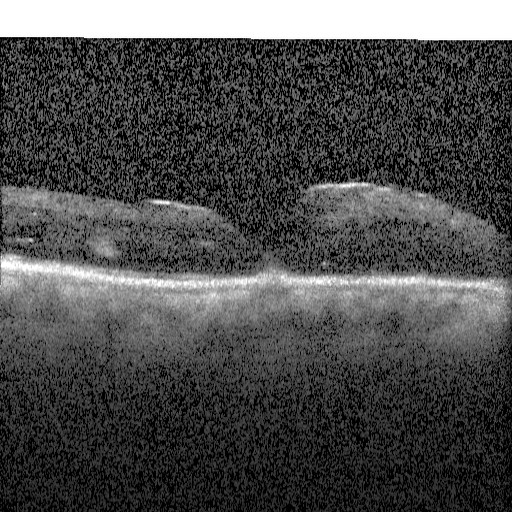

Optical coherence tomography B-scan; spectral-domain OCT
Assessment: DME.